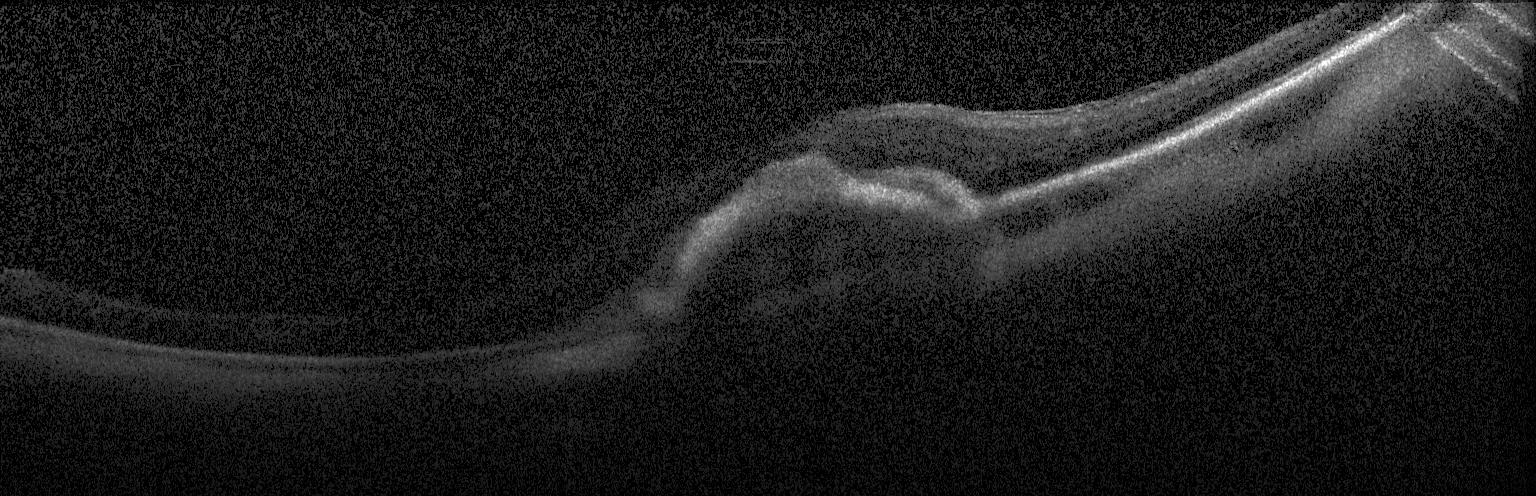 OCT finding: choroidal neovascularization (CNV).